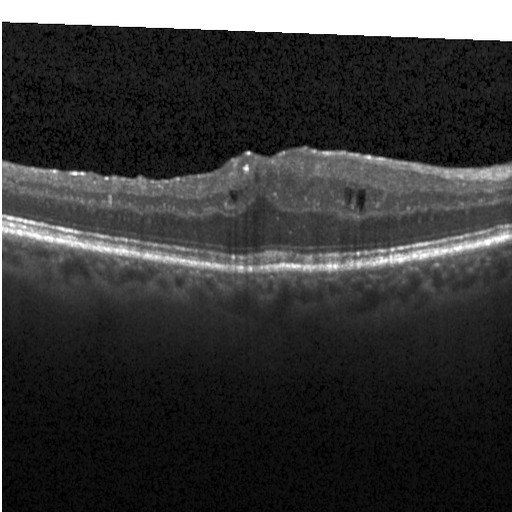

OCT line scan. Heidelberg Spectralis OCT system. Spectral-domain optical coherence tomography. Horizontal scan through the fovea. The scan shows diabetic macular edema (DME).